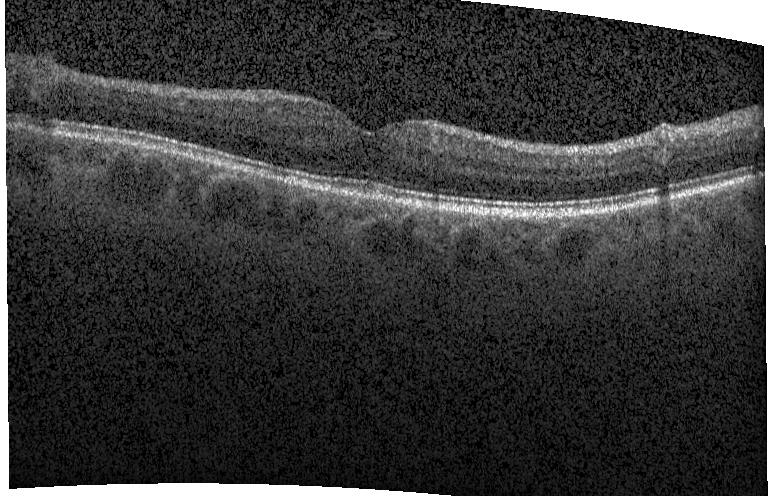

Impression: no choroidal neovascularization, diabetic macular edema, or drusen.